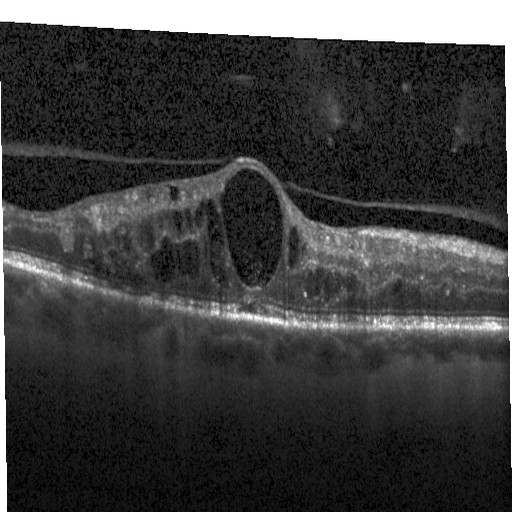 OCT B-scan showing diabetic macular edema (DME).